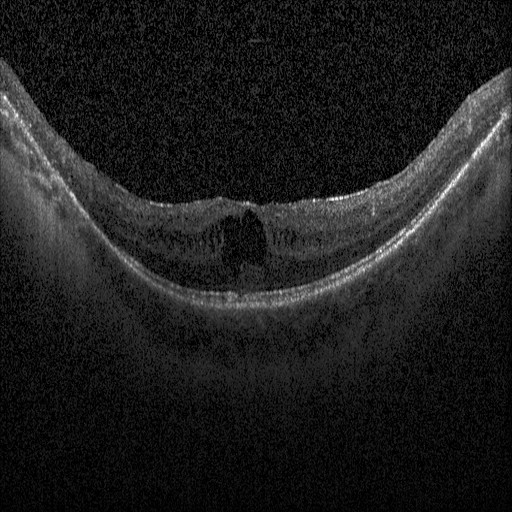 OCT line scan; spectral-domain OCT; through the macula; instrument: Heidelberg Spectralis. The scan shows diabetic macular edema.